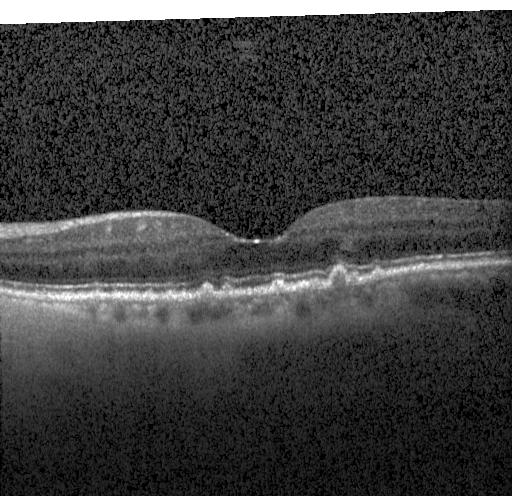 Optical coherence tomography scan.
Finding: drusen.